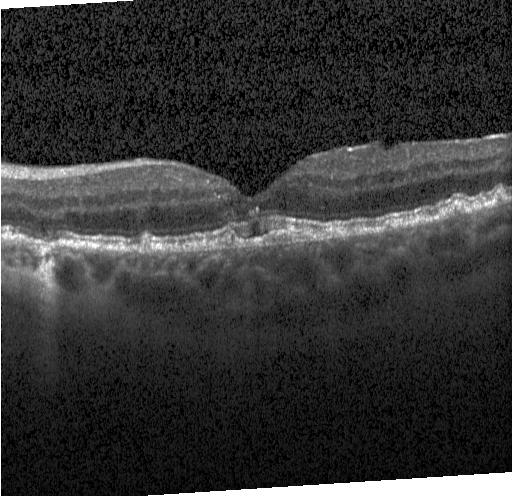 Diagnosis: a choroidal neovascular membrane.